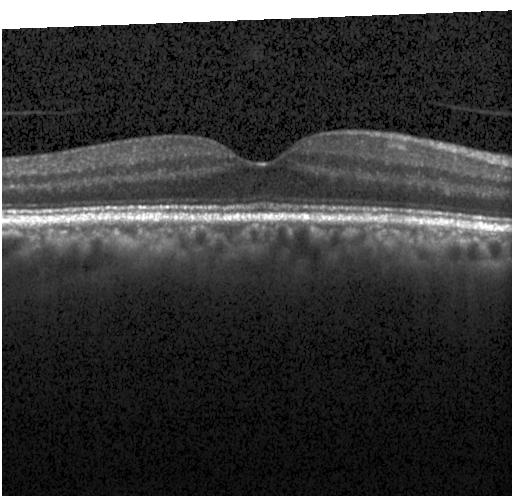 Optical coherence tomography B-scan, spectral-domain OCT, Heidelberg Spectralis OCT system, horizontal scan through the fovea. OCT finding: no choroidal neovascularization, diabetic macular edema, or drusen.